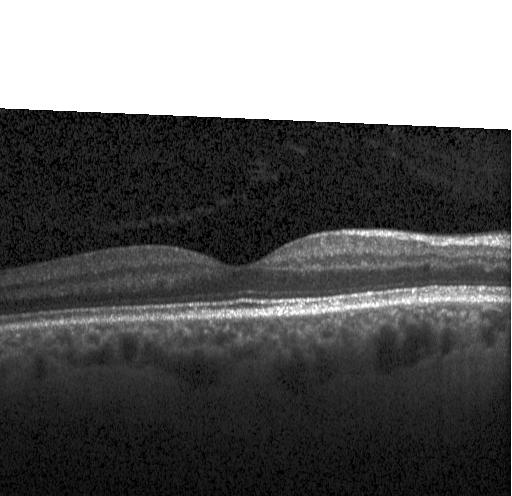
Dx: neither CNV, DME, nor drusen.